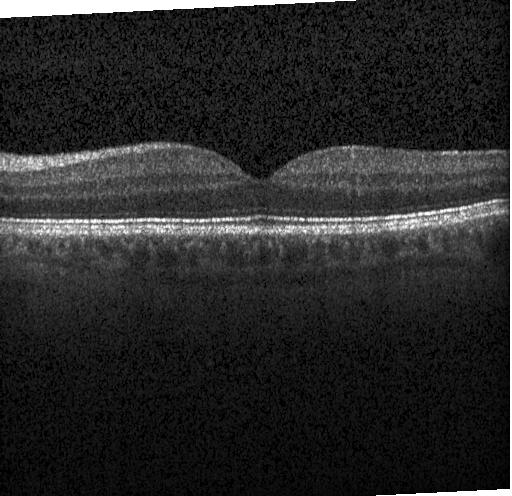
Optical coherence tomography scan; through the macula — Finding: no choroidal neovascularization, diabetic macular edema, or drusen.